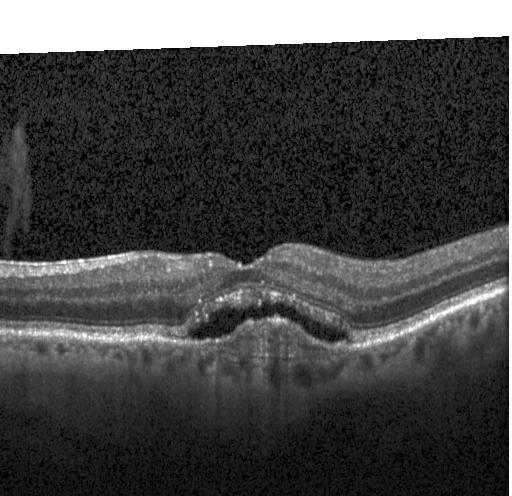

OCT line scan, Heidelberg Spectralis
Assessment: a choroidal neovascular membrane.